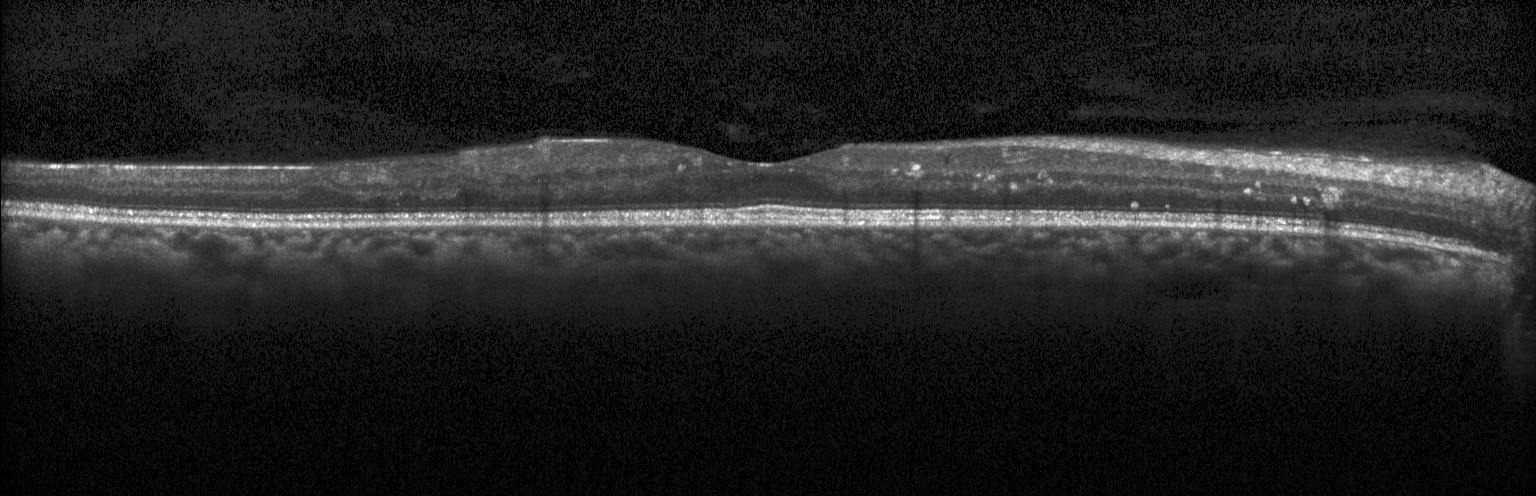 Instrument: Heidelberg Spectralis · optical coherence tomography B-scan · horizontal scan through the fovea · SD-OCT — The scan shows diabetic macular edema (DME).